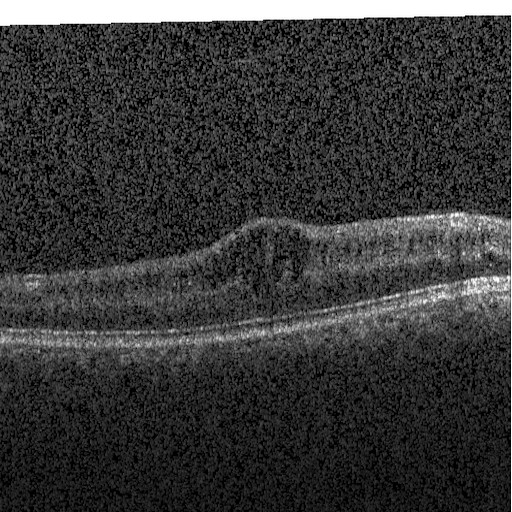

Assessment: diabetic macular edema (DME).